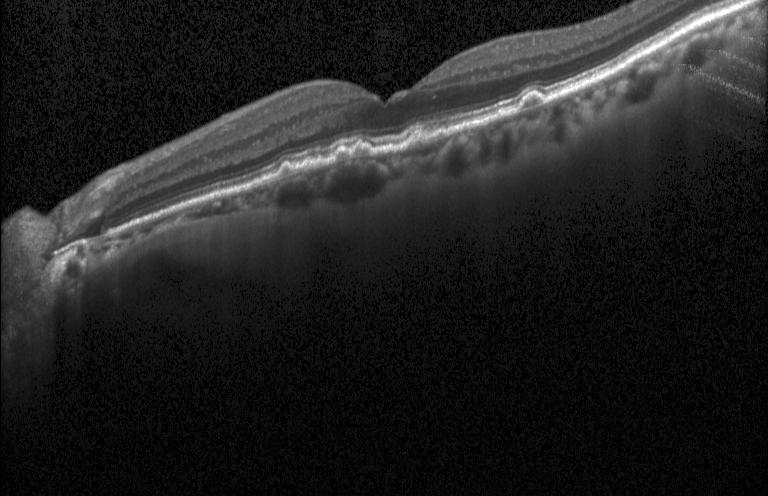 Spectral-domain OCT B-scan: drusen.